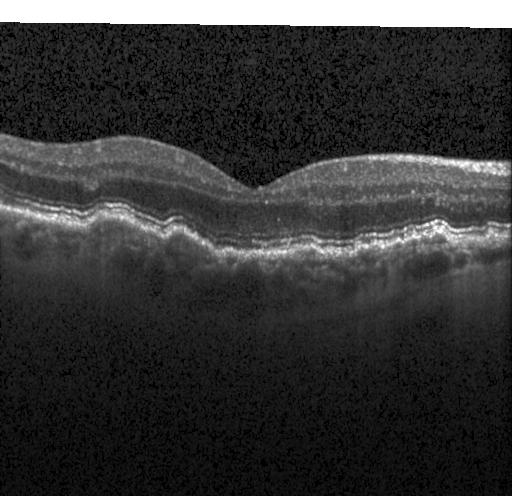

Spectral-domain optical coherence tomography; retinal OCT cross-section; centered on the fovea; Heidelberg Spectralis — Assessment: drusen.